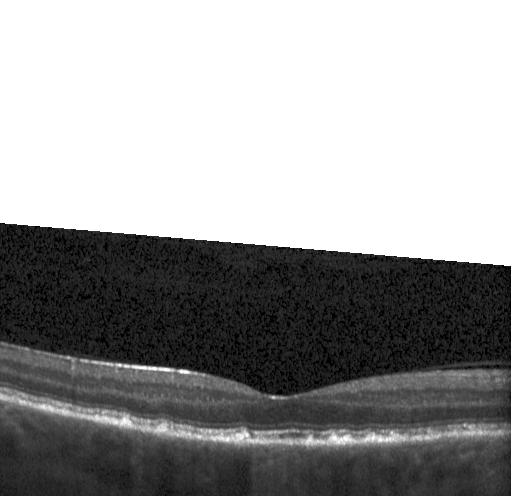
Finding: sub-RPE drusenoid deposits.